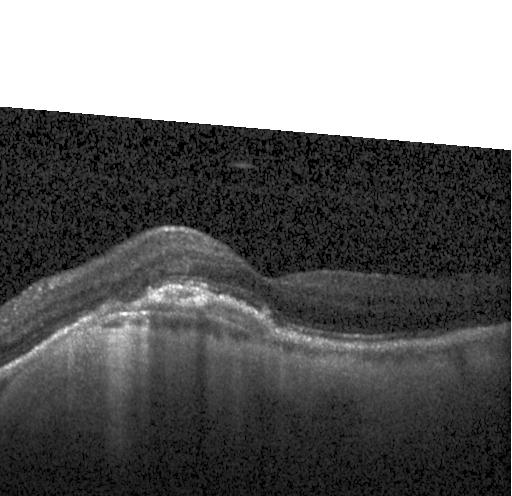

OCT B-scan showing choroidal neovascularization.